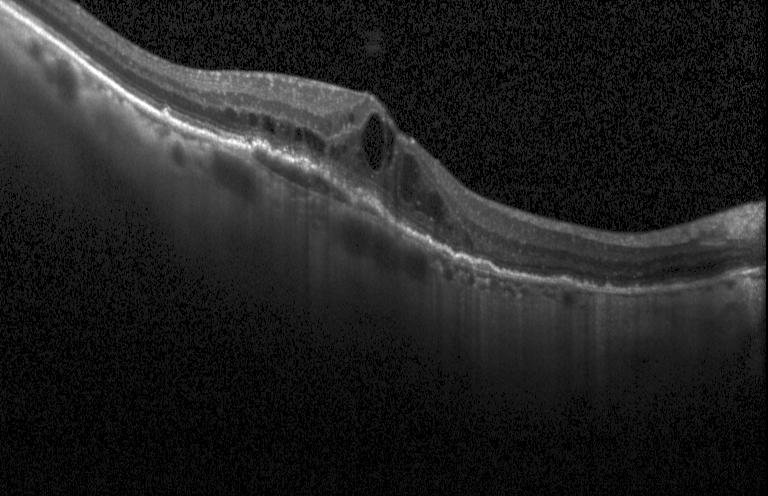

Optical coherence tomography B-scan; acquired on a Heidelberg Spectralis; horizontal scan through the fovea; spectral-domain OCT.
The scan shows choroidal neovascularization.